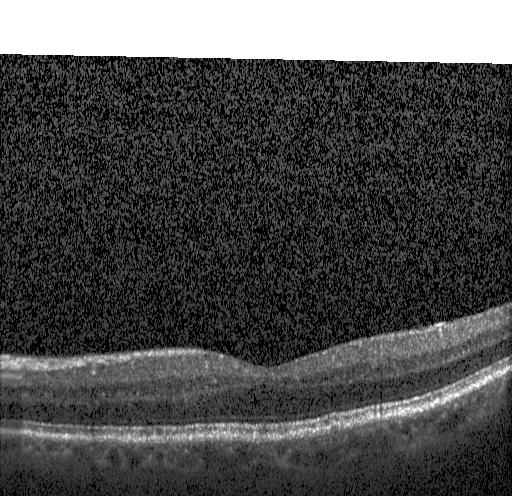

Spectral-domain OCT B-scan: no choroidal neovascularization, diabetic macular edema, or drusen.